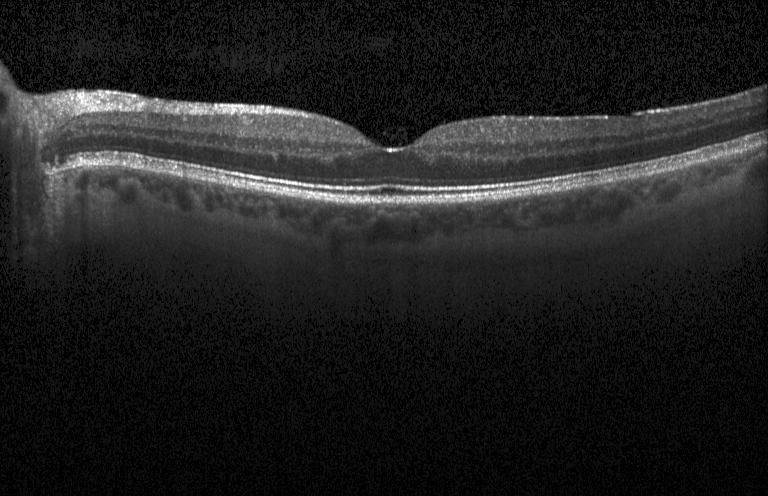
Fovea-centered · optical coherence tomography scan · Heidelberg Spectralis · SD-OCT — This B-scan demonstrates no evidence of CNV, DME, or drusen.